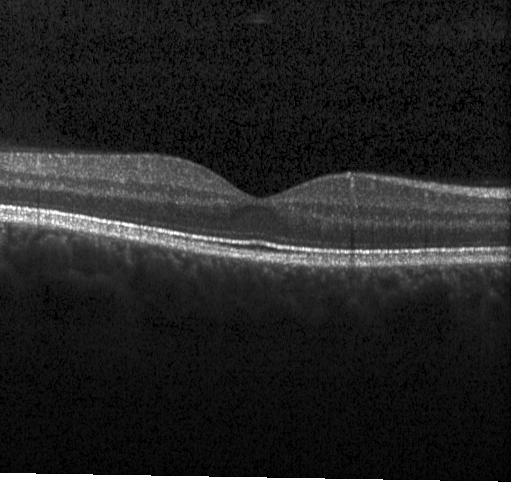

Spectral-domain OCT. OCT line scan.
OCT finding: neither CNV, DME, nor drusen.